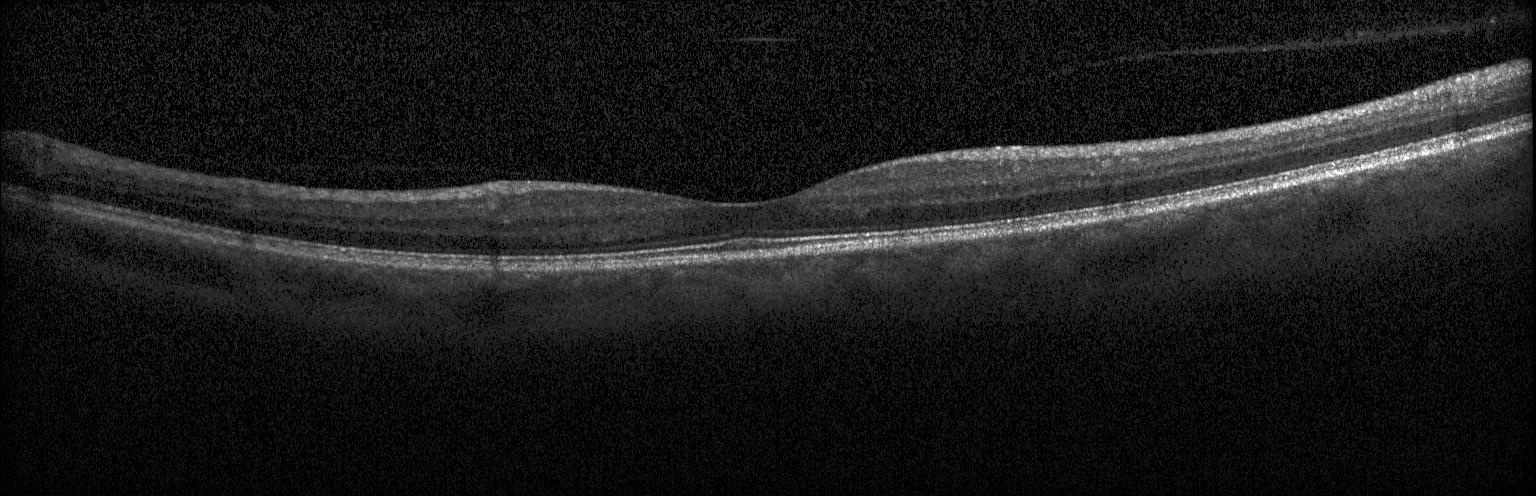

Heidelberg Spectralis OCT system. Retinal OCT B-scan. Horizontal scan through the fovea. SD-OCT — Macular OCT: no choroidal neovascularization, diabetic macular edema, or drusen.